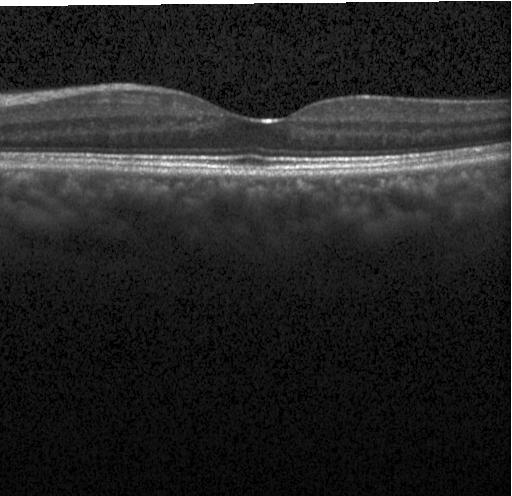
Diagnosis: no evidence of choroidal neovascularization, diabetic macular edema, or drusen.